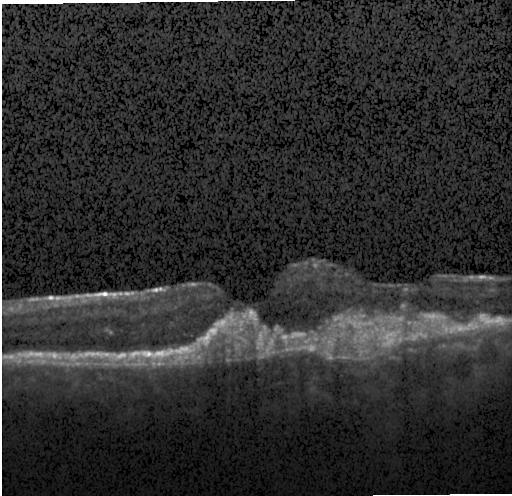 Assessment: CNV.